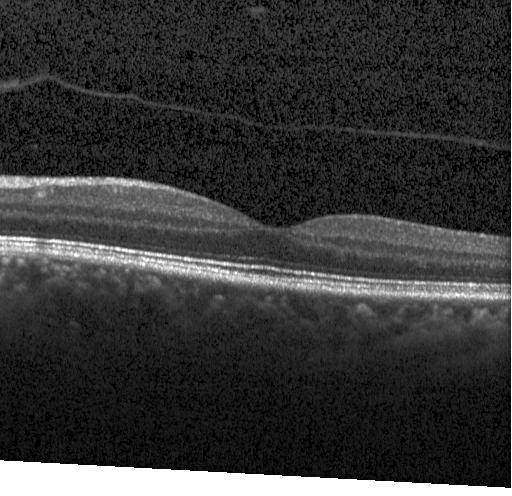
Finding: no choroidal neovascularization, no diabetic macular edema, and no drusen.